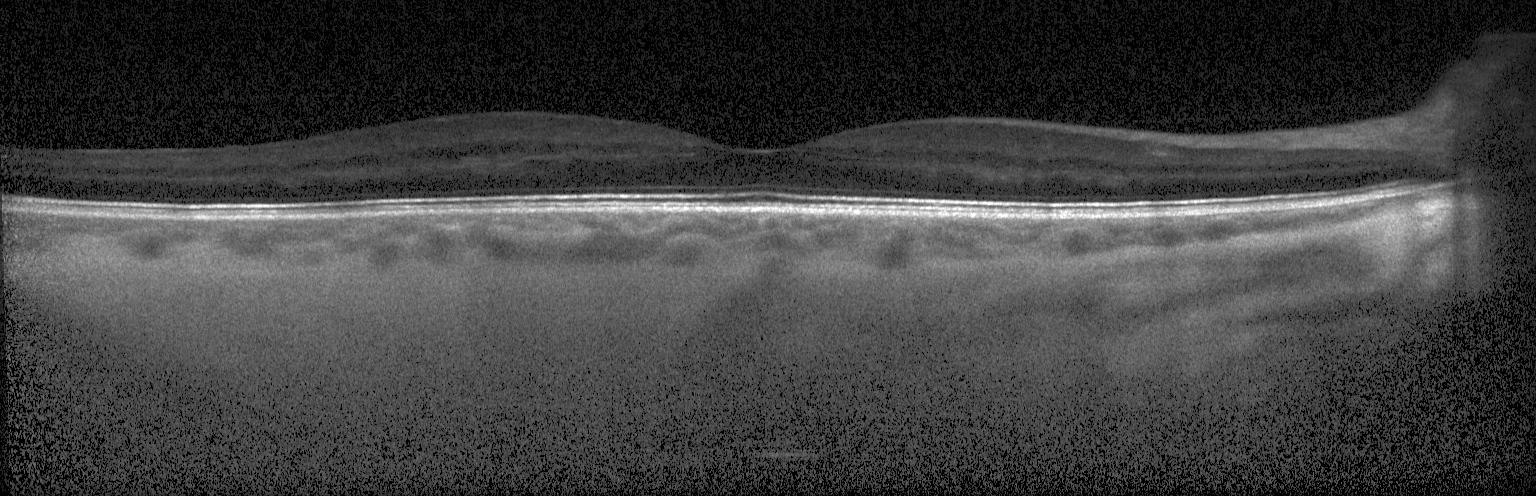
OCT line scan
Finding: no choroidal neovascularization, diabetic macular edema, or drusen.